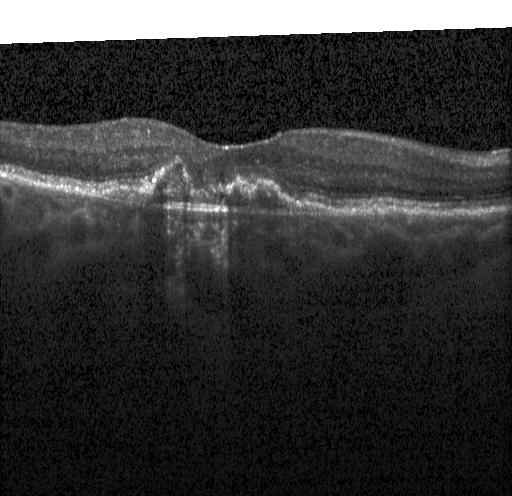
OCT line scan — Impression: choroidal neovascularization.